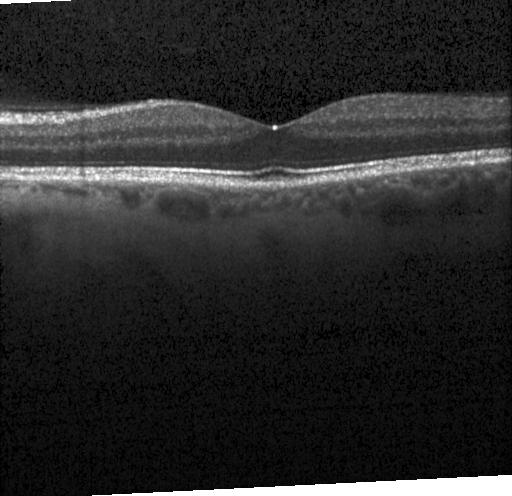

Optical coherence tomography scan.
Finding: no evidence of CNV, DME, or drusen.